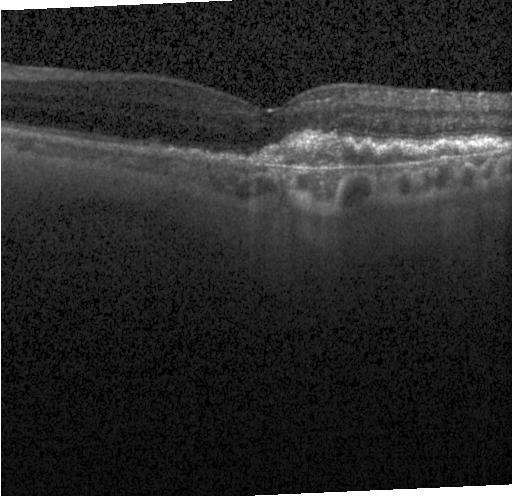 Optical coherence tomography B-scan; spectral-domain optical coherence tomography — Diagnosis: a choroidal neovascular membrane.